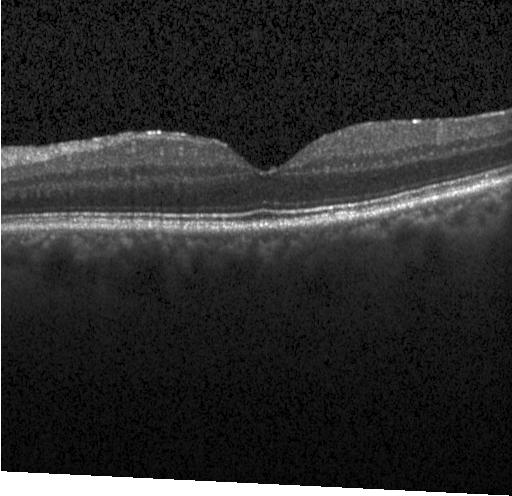

OCT line scan.
Assessment: neither CNV, DME, nor drusen.